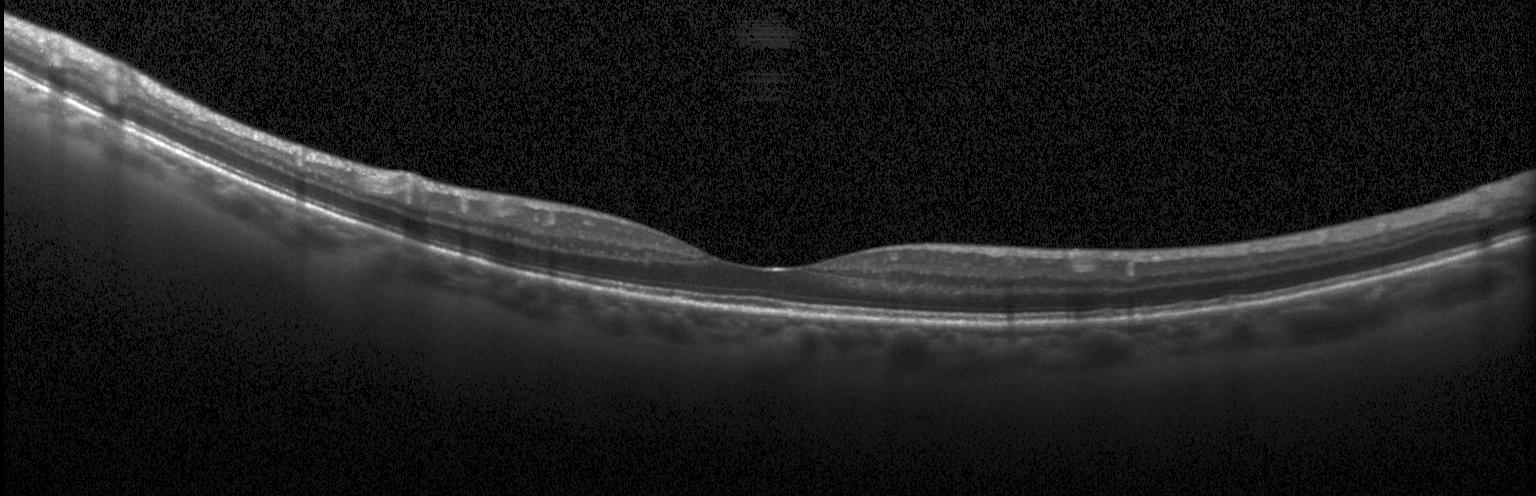
Impression: no evidence of choroidal neovascularization, diabetic macular edema, or drusen.